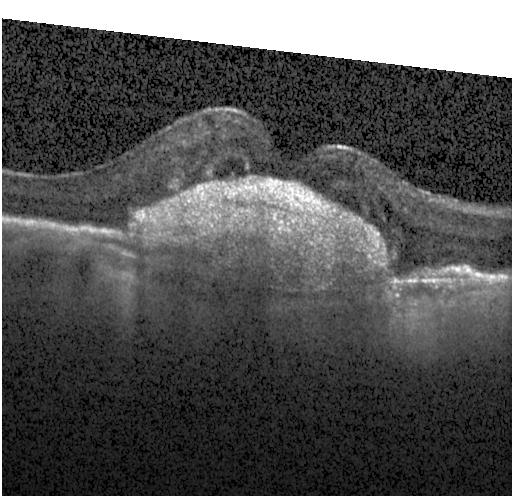

Retinal OCT B-scan; Heidelberg Spectralis OCT system. Diagnosis: a choroidal neovascular membrane.